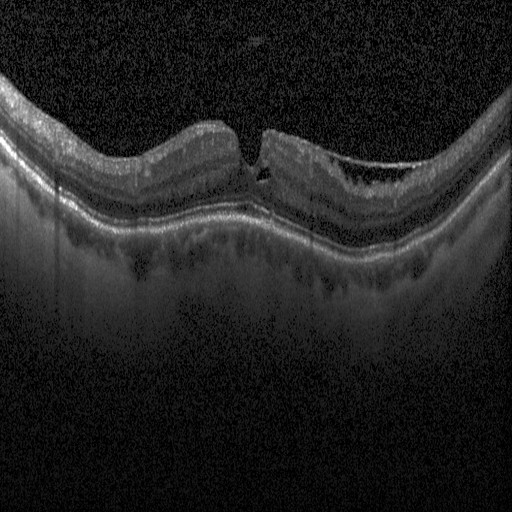 Diagnosis: diabetic macular edema (DME).